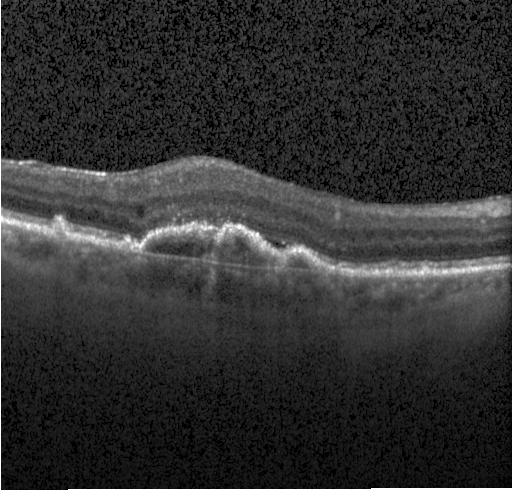
Fovea-centered; retinal OCT cross-section.
Choroidal neovascularization (CNV).